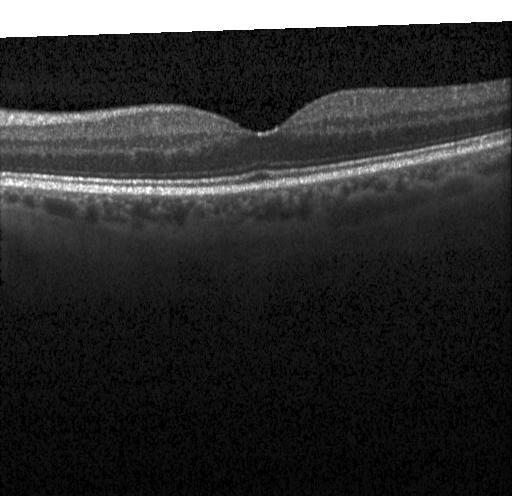

OCT finding: no evidence of CNV, DME, or drusen.